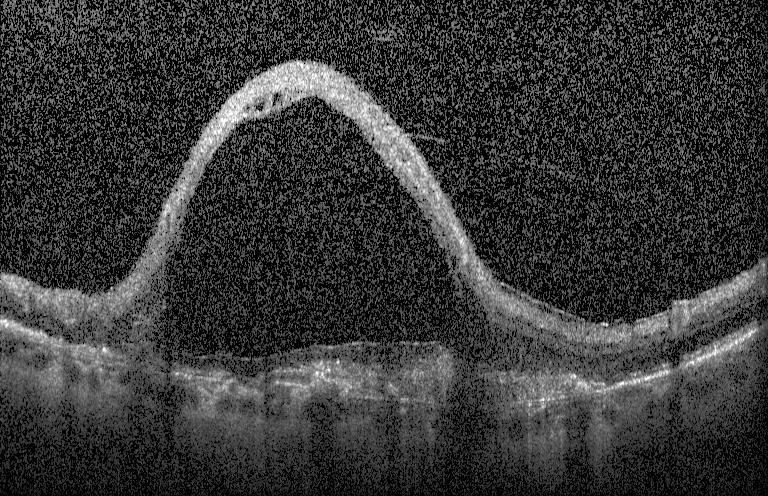

OCT B-scan; horizontal scan through the fovea; spectral-domain OCT.
Diagnosis: a choroidal neovascular membrane.